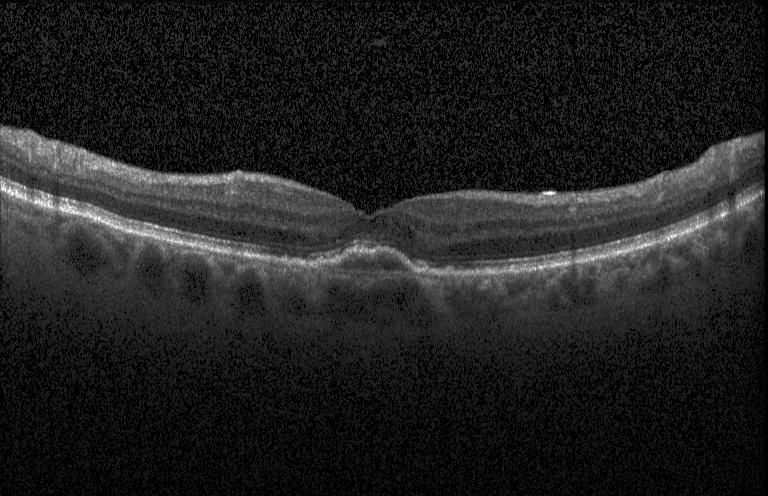
Optical coherence tomography B-scan, SD-OCT. Finding: a choroidal neovascular membrane.